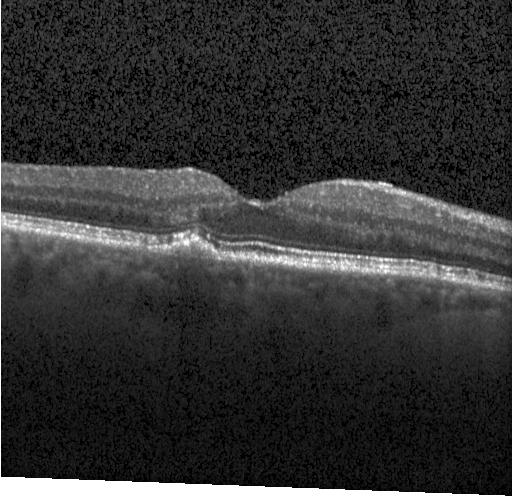 OCT line scan; acquired on a Heidelberg Spectralis; horizontal scan through the fovea
This B-scan demonstrates sub-RPE drusenoid deposits.